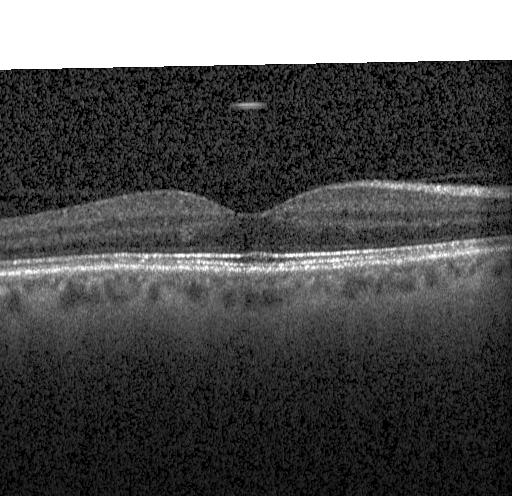
Spectral-domain optical coherence tomography; Heidelberg Spectralis; optical coherence tomography scan
Finding: no choroidal neovascularization, diabetic macular edema, or drusen.